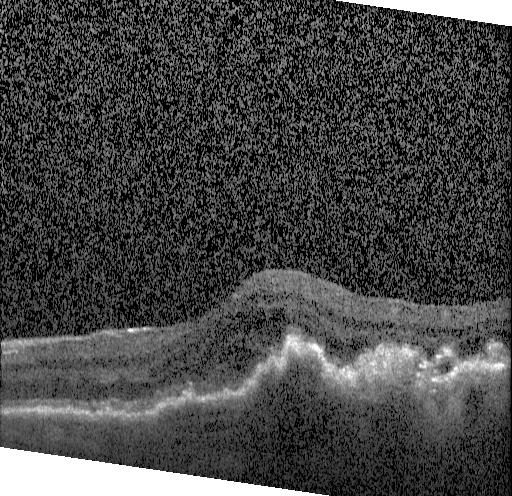
Fovea-centered, optical coherence tomography scan, Heidelberg Spectralis OCT system.
Impression: CNV.